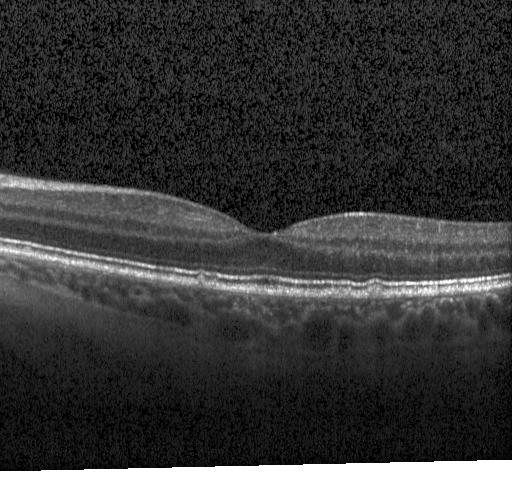

OCT B-scan showing drusen.